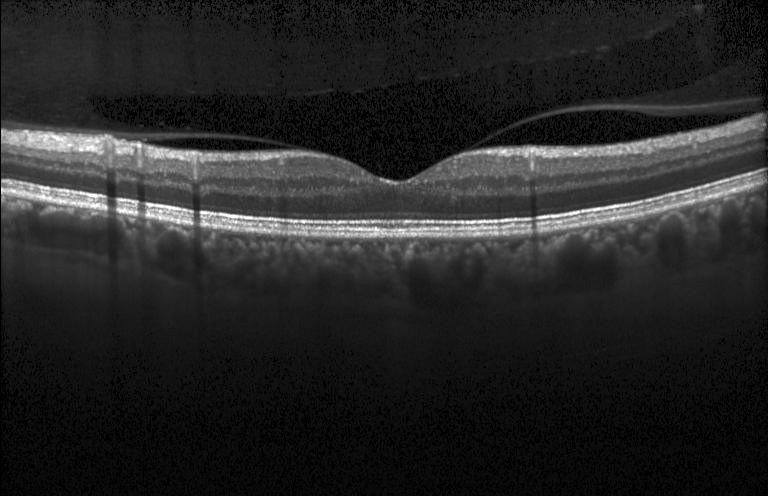
Spectral-domain optical coherence tomography; centered on the fovea; Heidelberg Spectralis OCT system; OCT B-scan — Neither CNV, DME, nor drusen.